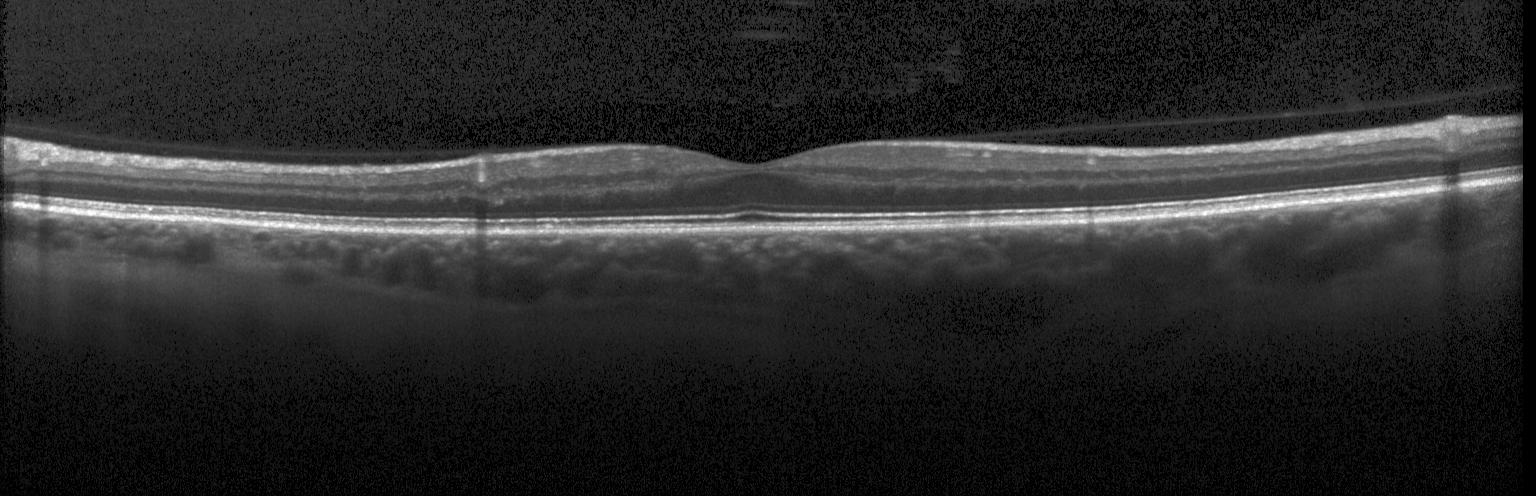
OCT finding: neither CNV, DME, nor drusen.